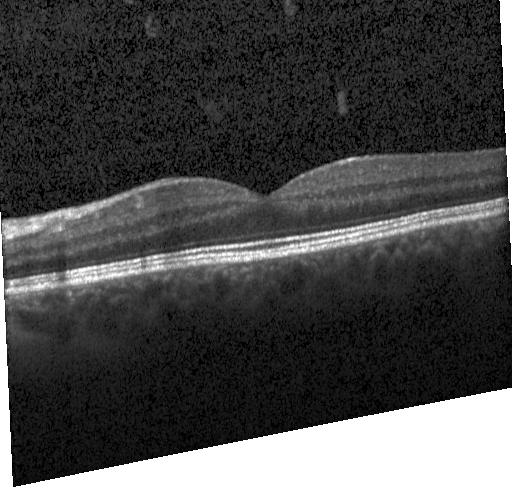
Spectral-domain OCT B-scan: no choroidal neovascularization, diabetic macular edema, or drusen.